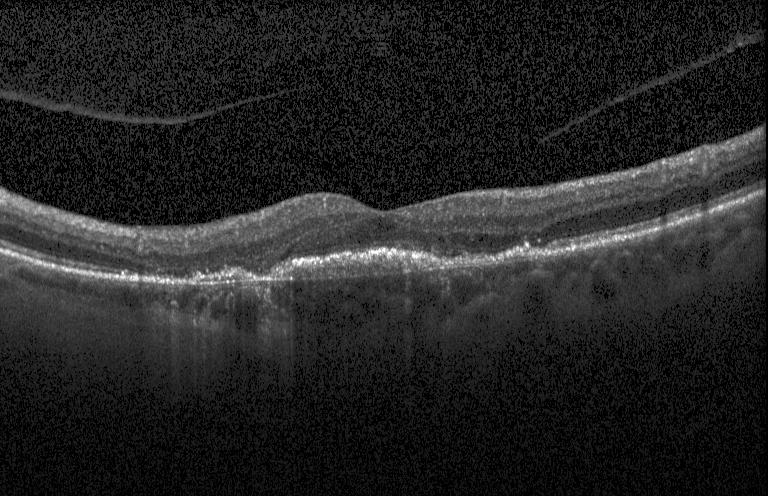 Diagnosis: choroidal neovascularization (CNV).